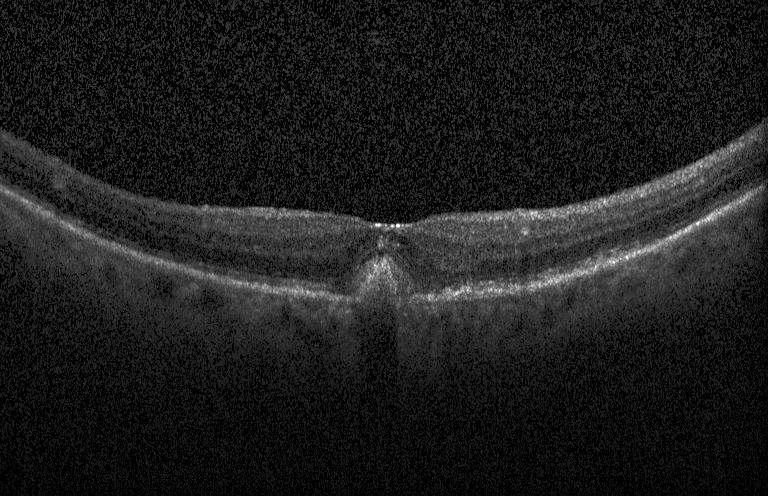

Spectral-domain OCT B-scan: a choroidal neovascular membrane.